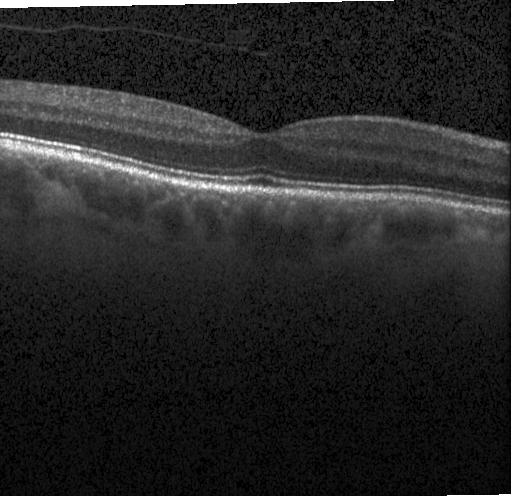 Spectral-domain OCT · OCT line scan
Assessment: no evidence of choroidal neovascularization, diabetic macular edema, or drusen.